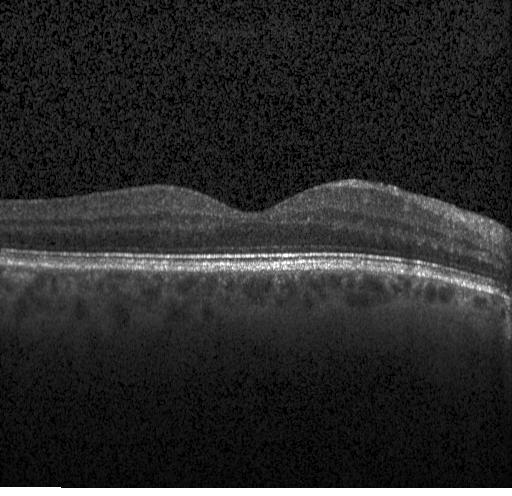

Optical coherence tomography B-scan — OCT finding: no CNV, no DME, and no drusen.